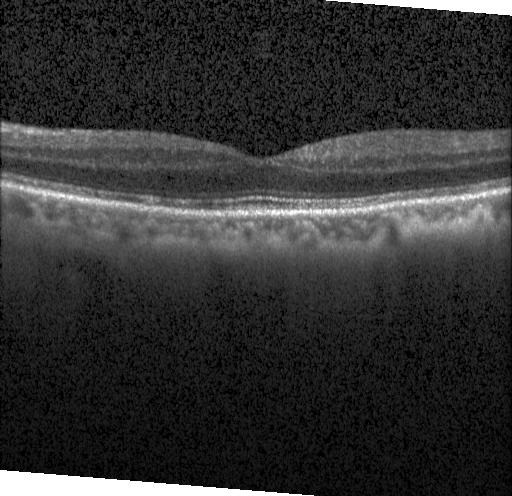
Retinal OCT cross-section. Dx: no evidence of choroidal neovascularization, diabetic macular edema, or drusen.